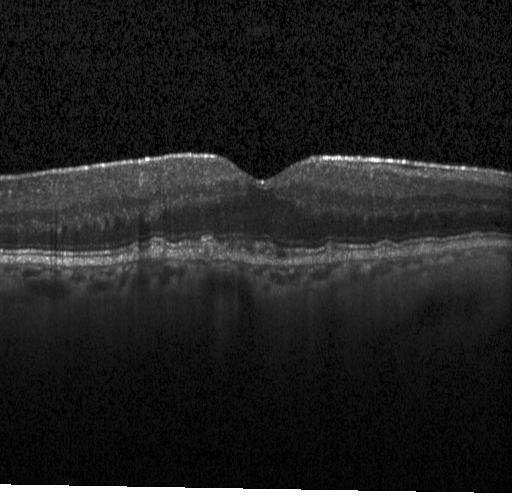 OCT finding: sub-RPE drusenoid deposits.